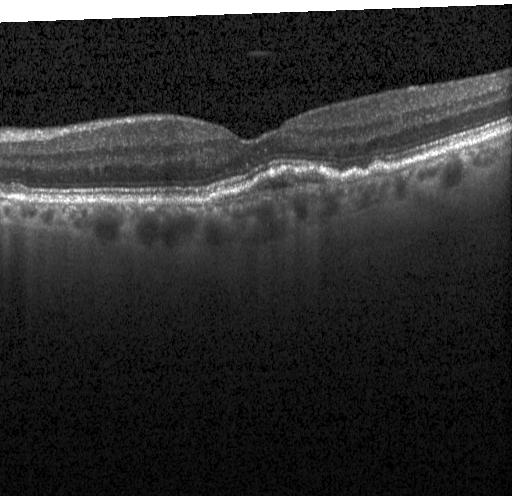
Optical coherence tomography scan, spectral-domain OCT, centered on the fovea — Finding: a choroidal neovascular membrane.